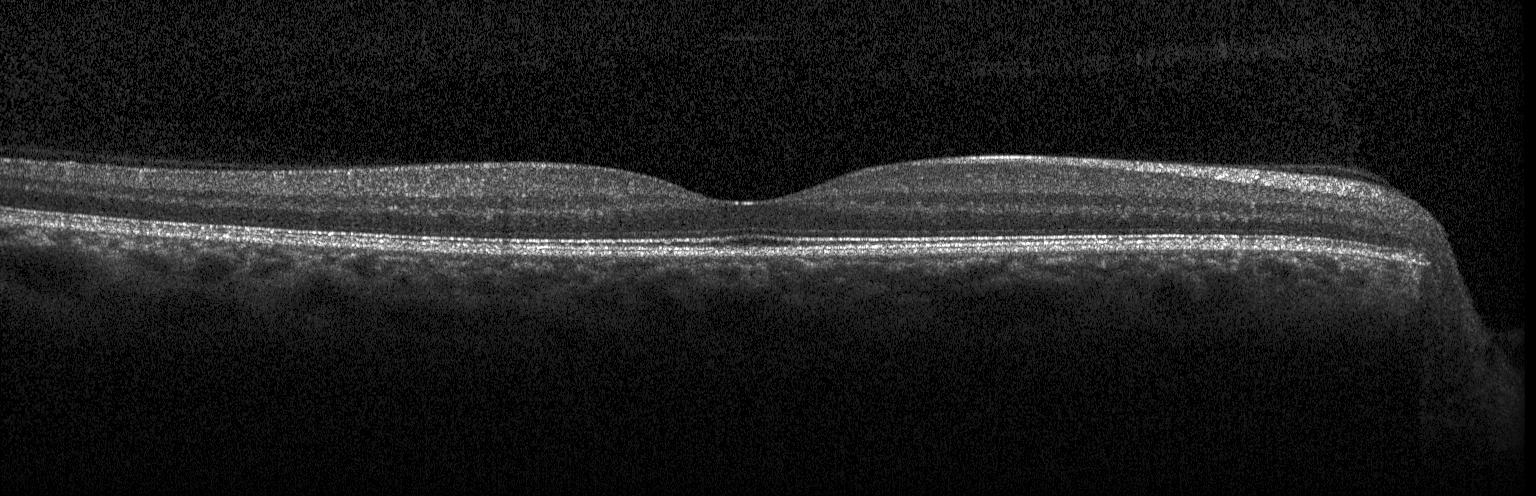

OCT finding: no evidence of CNV, DME, or drusen.